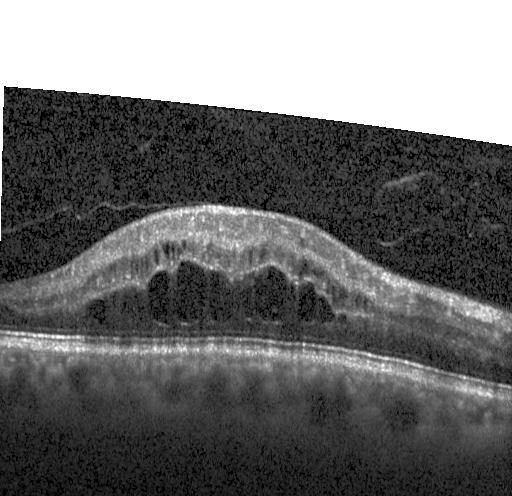 OCT line scan. Diabetic macular edema.